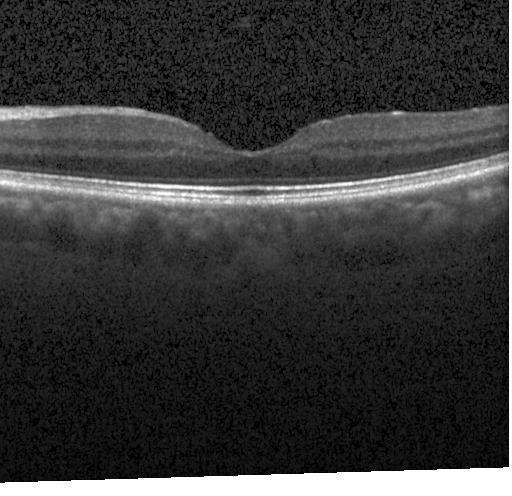
Centered on the fovea · spectral-domain OCT · optical coherence tomography B-scan · acquired on a Heidelberg Spectralis.
OCT finding: no evidence of choroidal neovascularization, diabetic macular edema, or drusen.